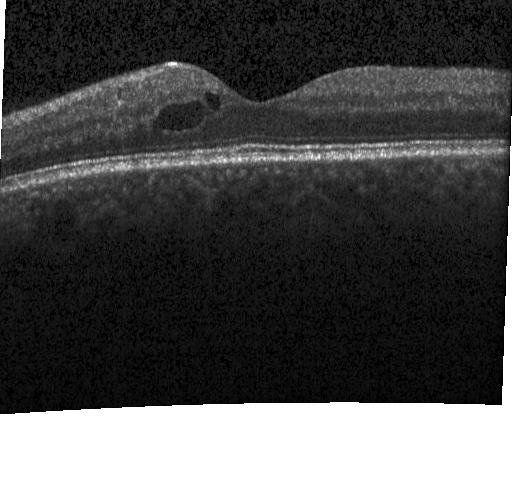

OCT B-scan showing DME.